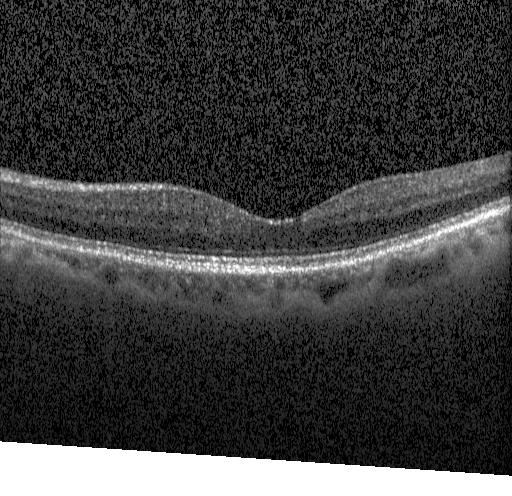 OCT B-scan showing no CNV, no DME, and no drusen.